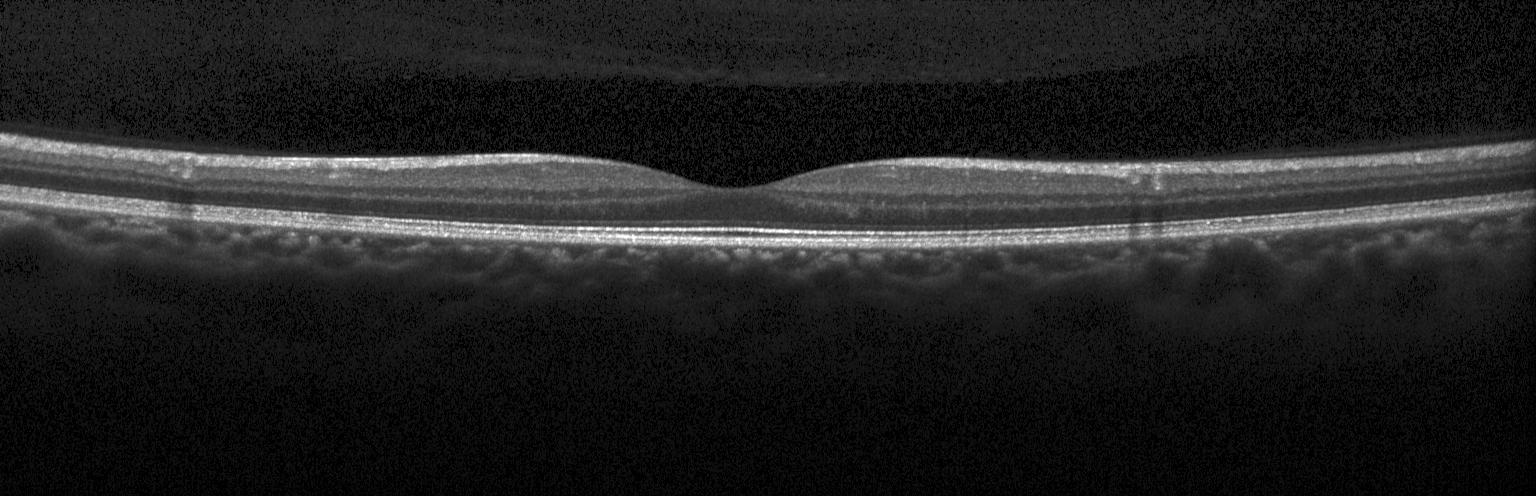

Acquired on a Heidelberg Spectralis, fovea-centered, OCT B-scan — Assessment: no choroidal neovascularization, diabetic macular edema, or drusen.